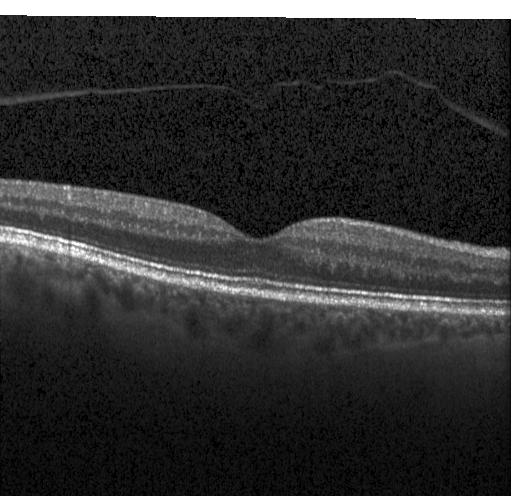

Retinal OCT cross-section, spectral-domain optical coherence tomography — Impression: no evidence of CNV, DME, or drusen.